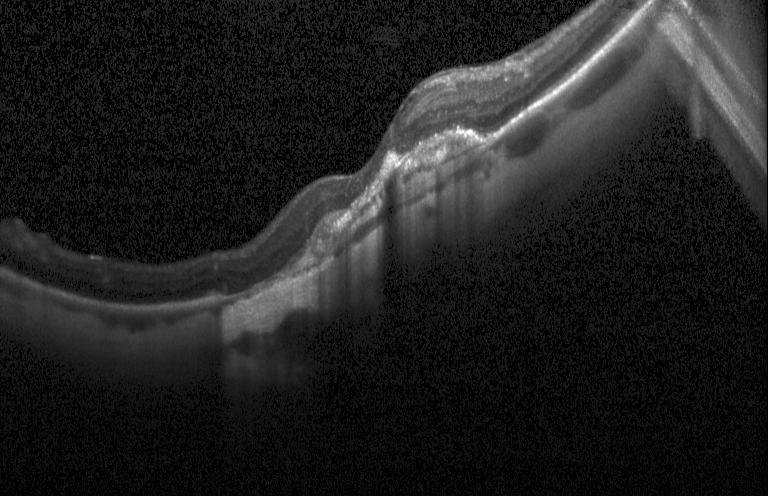
Heidelberg Spectralis OCT system; macular scan; retinal OCT B-scan. Assessment: a choroidal neovascular membrane.